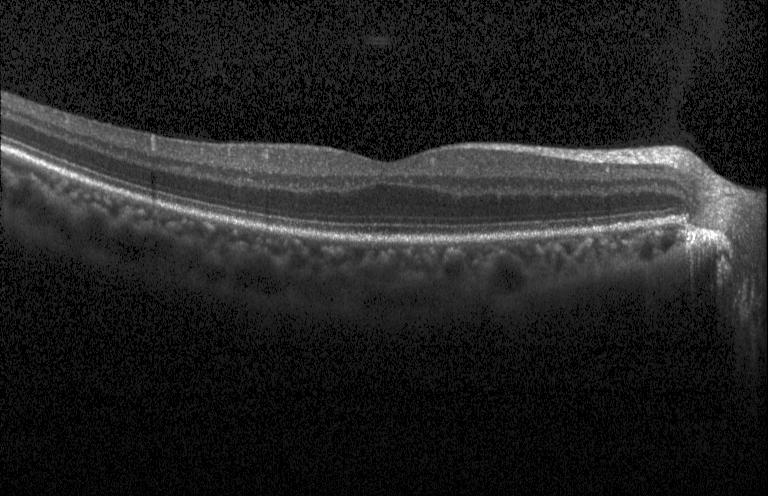
Diagnosis: no choroidal neovascularization, no diabetic macular edema, and no drusen.